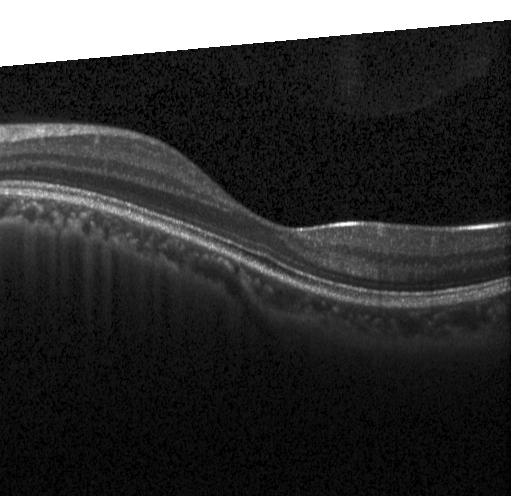 Retinal OCT B-scan.
Impression: no choroidal neovascularization, no diabetic macular edema, and no drusen.